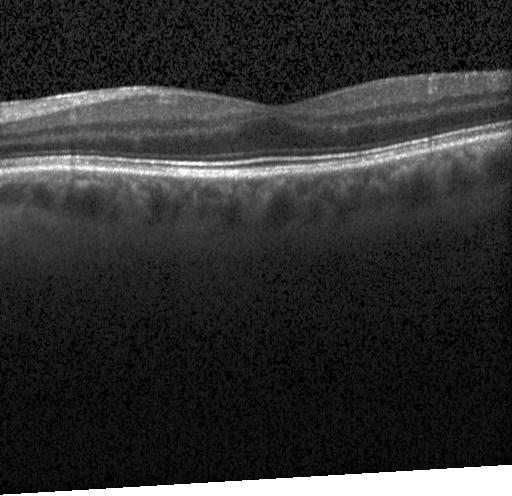

Acquired on a Heidelberg Spectralis · macular scan · retinal OCT cross-section — This B-scan demonstrates no CNV, no DME, and no drusen.